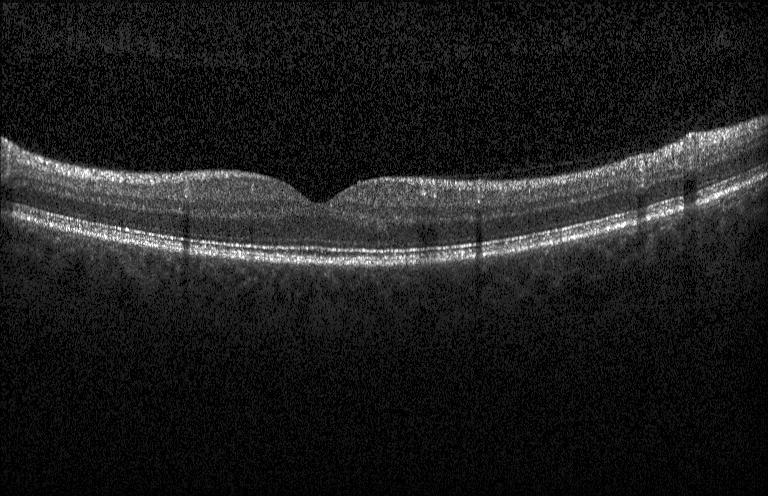
OCT B-scan.
This B-scan demonstrates neither CNV, DME, nor drusen.